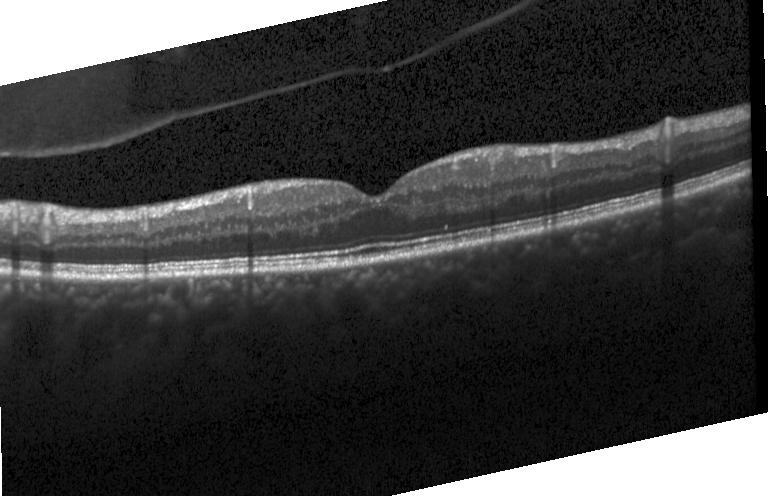 Instrument: Heidelberg Spectralis; optical coherence tomography B-scan; spectral-domain optical coherence tomography
Impression: no choroidal neovascularization, diabetic macular edema, or drusen.